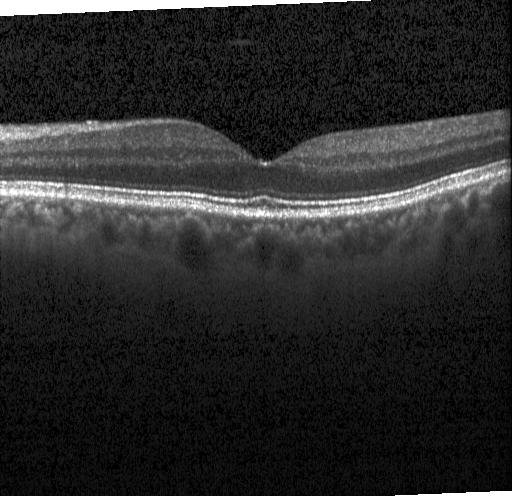

Dx: no choroidal neovascularization, diabetic macular edema, or drusen.